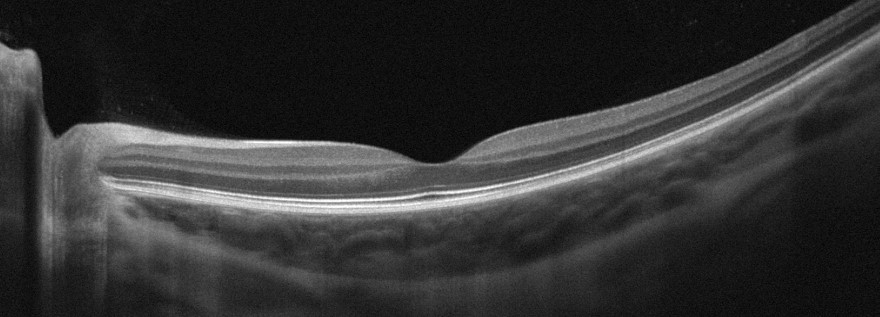 Instrument: Optovue Avanti RTVue XR; fovea-centered; retinal OCT cross-section
OCT finding: absence of AMD, DME, ERM, RAO, RVO, and vitreomacular interface disease.